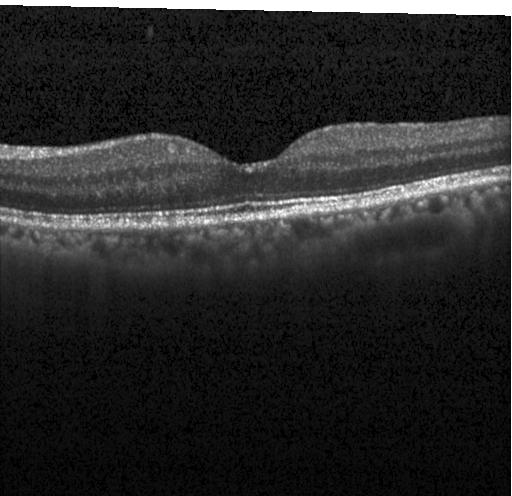
OCT B-scan
Impression: no evidence of choroidal neovascularization, diabetic macular edema, or drusen.